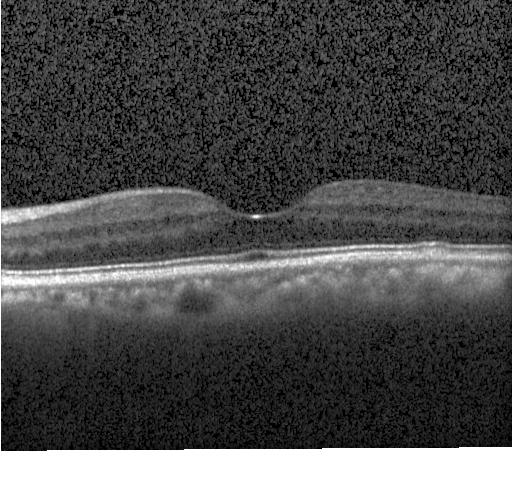

Horizontal scan through the fovea, optical coherence tomography B-scan
Diagnosis: no choroidal neovascularization, diabetic macular edema, or drusen.